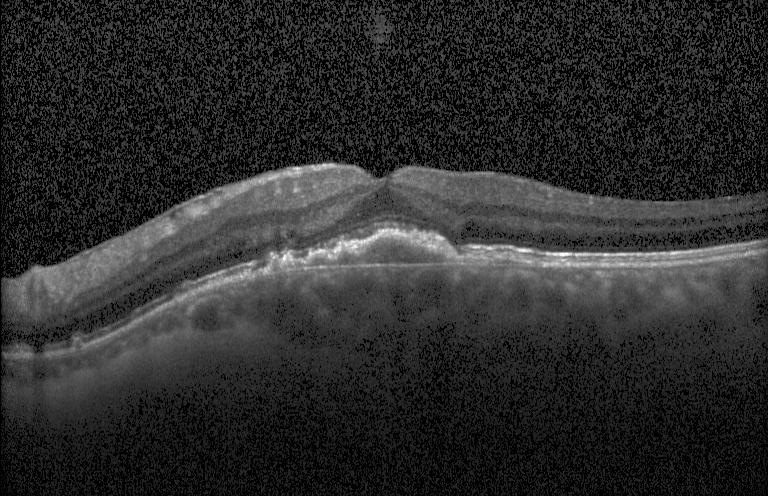
OCT B-scan.
Impression: a choroidal neovascular membrane.